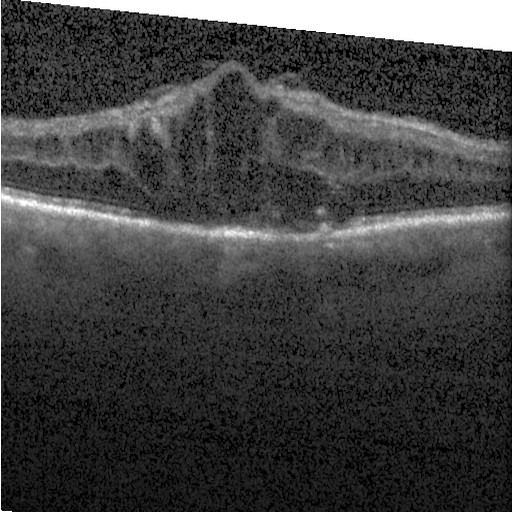

Finding: DME.